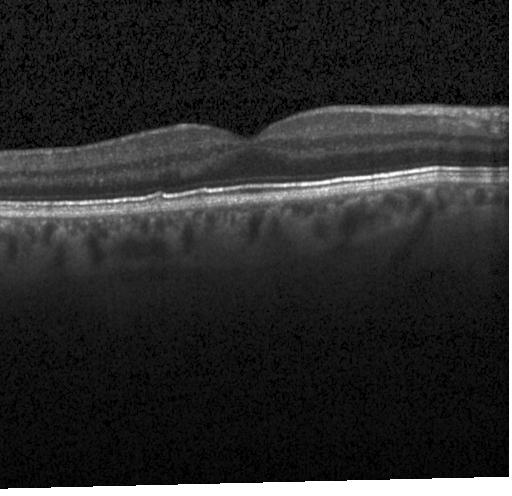

OCT finding: drusen.